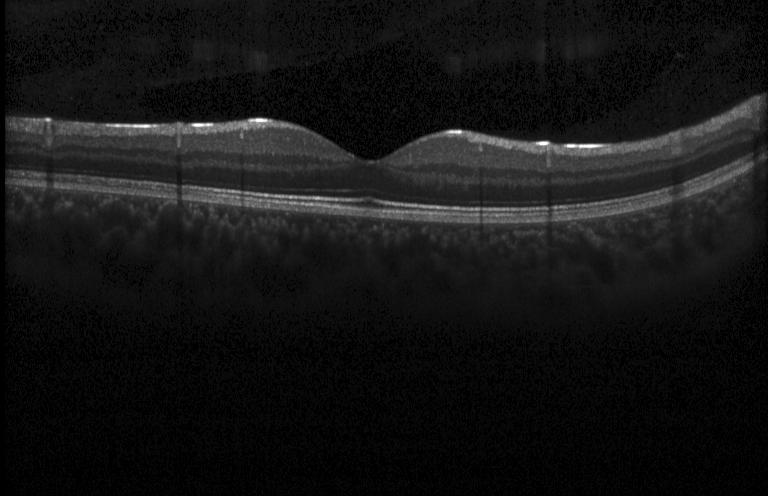 OCT line scan.
This B-scan demonstrates no choroidal neovascularization, diabetic macular edema, or drusen.